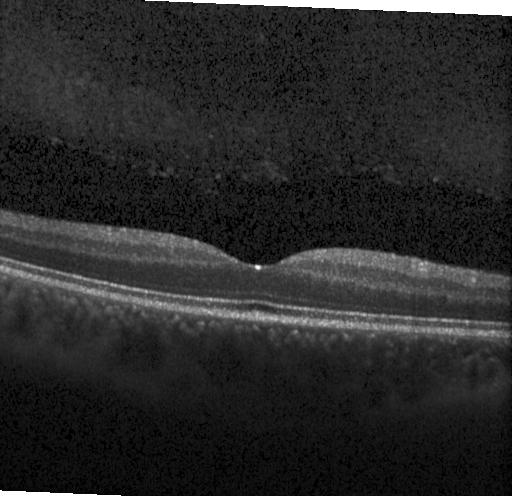

Spectral-domain optical coherence tomography · Heidelberg Spectralis OCT system · OCT line scan.
Finding: neither choroidal neovascularization, diabetic macular edema, nor drusen.